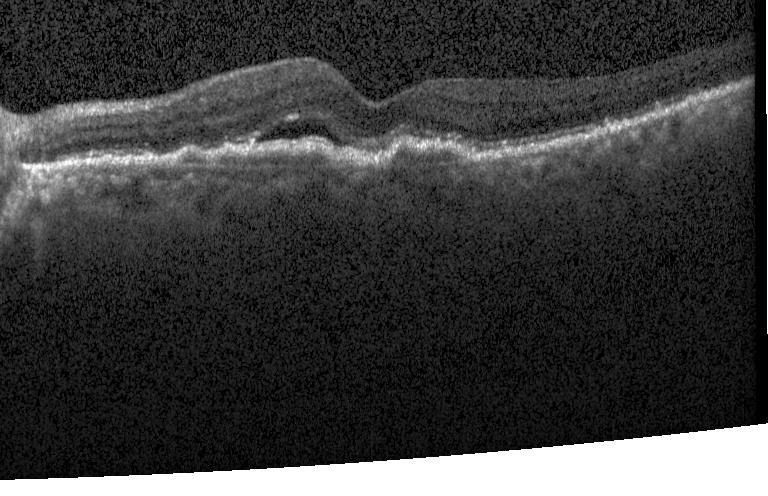

Assessment: a choroidal neovascular membrane.